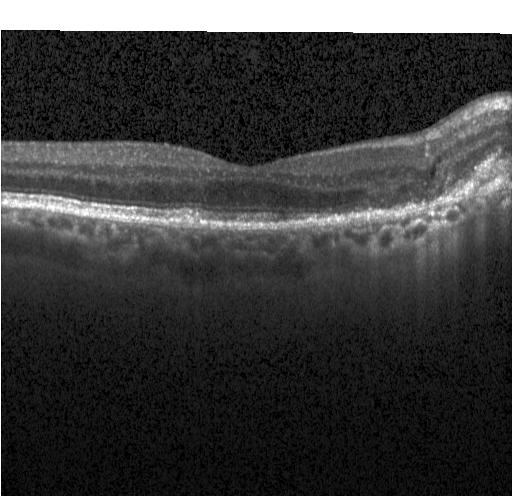

Optical coherence tomography B-scan. Macular scan. Dx: a choroidal neovascular membrane.